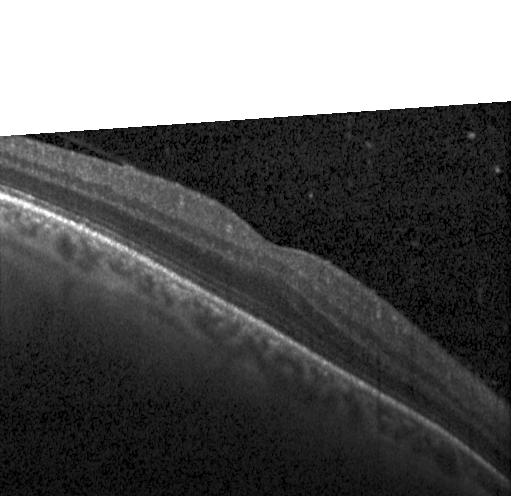

OCT scan showing neither choroidal neovascularization, diabetic macular edema, nor drusen.